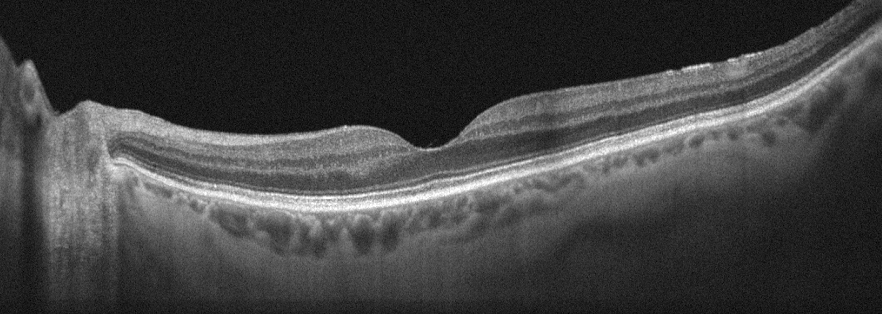
Retinal OCT B-scan; OS. Assessment: no AMD, DME, ERM, RAO, RVO, or VID.